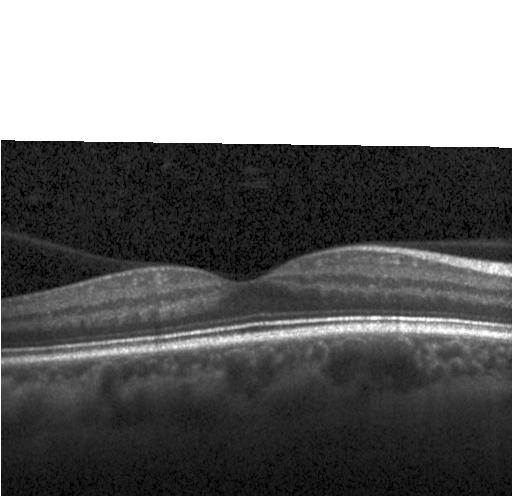
Optical coherence tomography scan; instrument: Heidelberg Spectralis; centered on the fovea. Dx: no CNV, DME, or drusen.